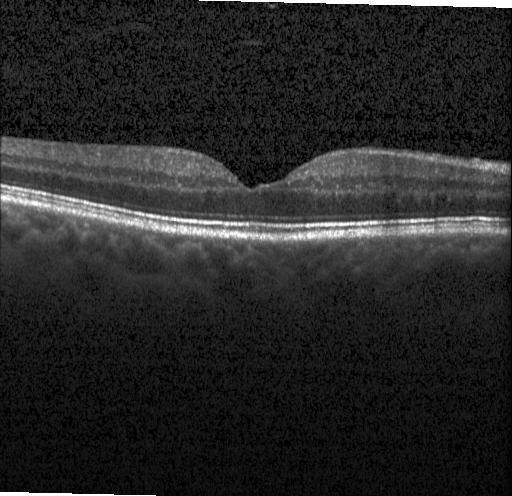

Retinal OCT cross-section. Neither CNV, DME, nor drusen.